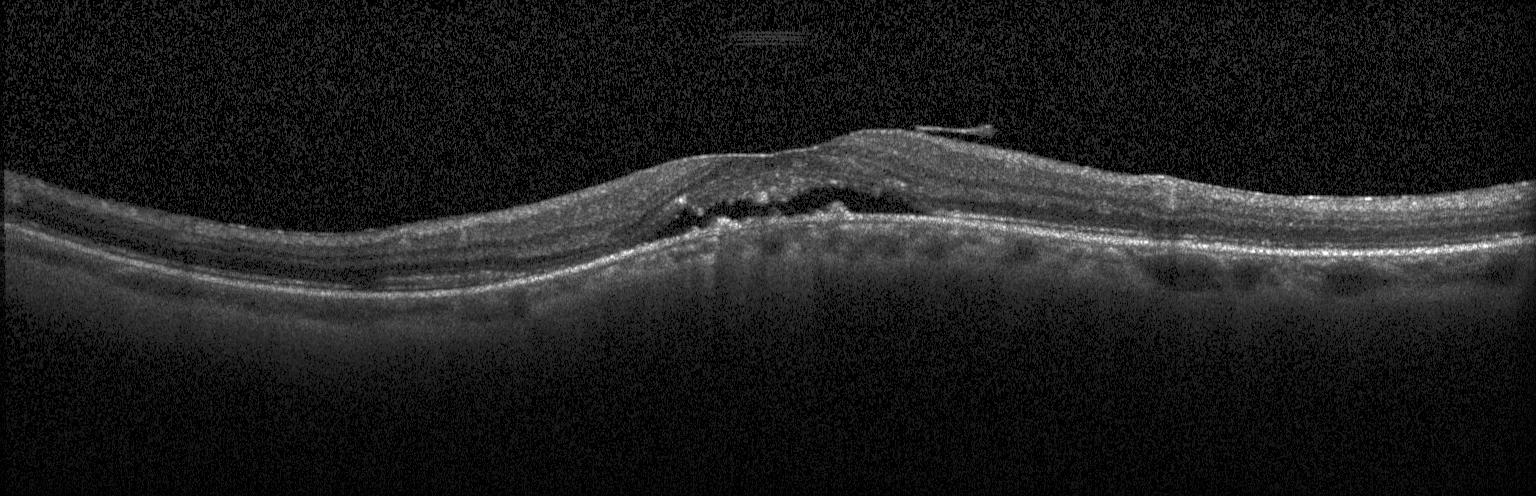
Optical coherence tomography scan; acquired on a Heidelberg Spectralis; centered on the fovea. Finding: choroidal neovascularization (CNV).